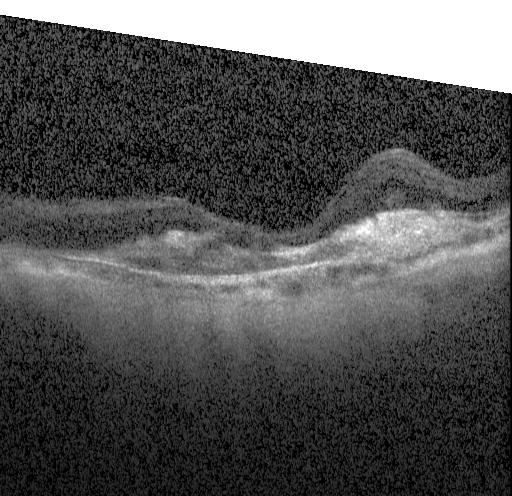 Heidelberg Spectralis · optical coherence tomography B-scan · through the macula — Assessment: a choroidal neovascular membrane.